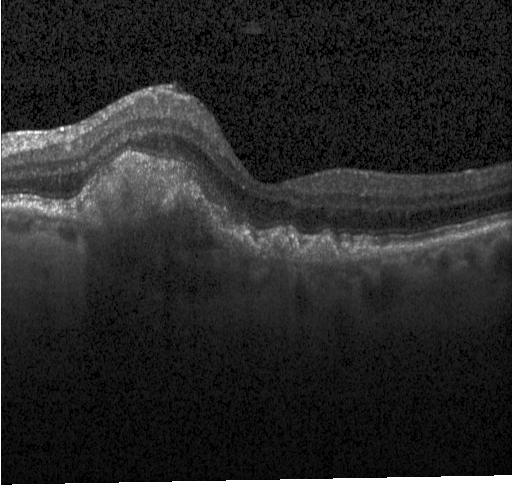

Centered on the fovea, retinal OCT cross-section, Heidelberg Spectralis OCT system, SD-OCT.
Macular OCT: CNV.